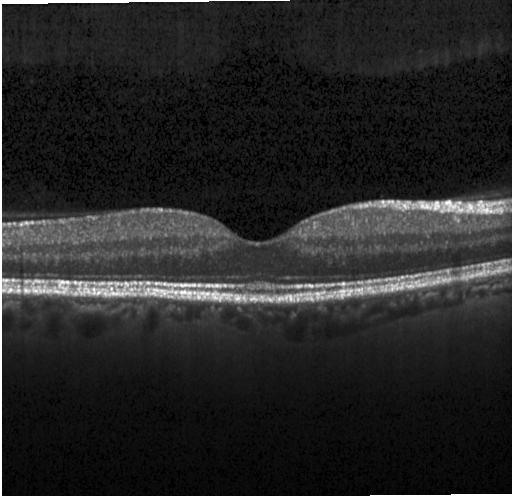
Retinal OCT B-scan — Diagnosis: no choroidal neovascularization, diabetic macular edema, or drusen.